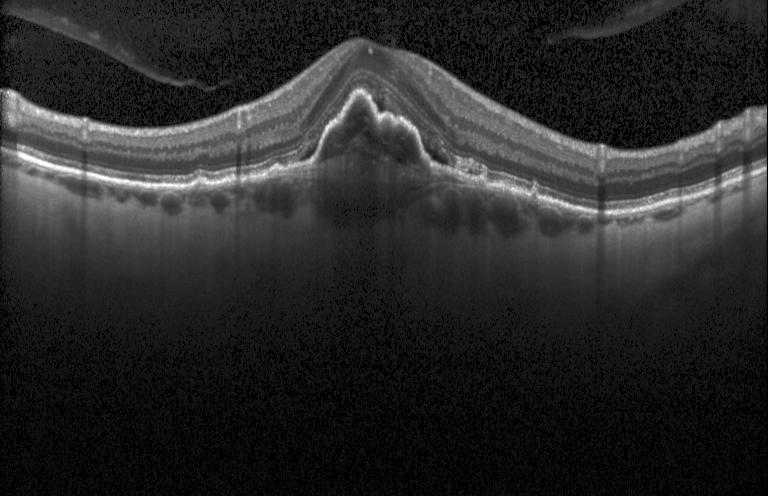
Retinal OCT cross-section. Impression: CNV.